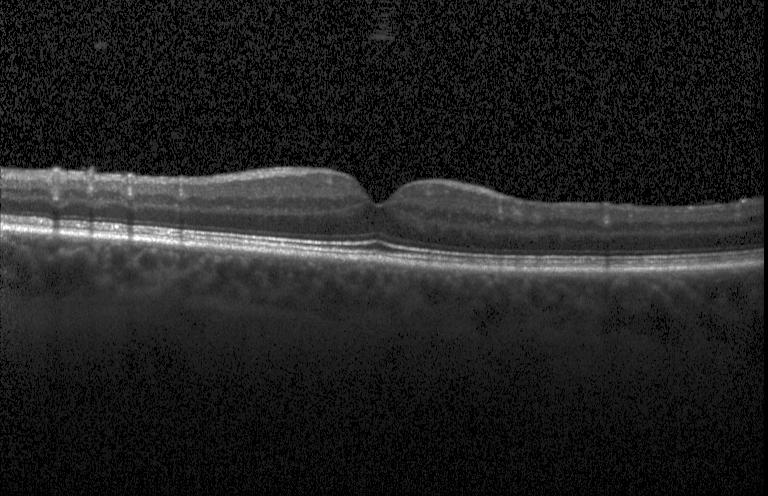

Macular OCT: no choroidal neovascularization, diabetic macular edema, or drusen.